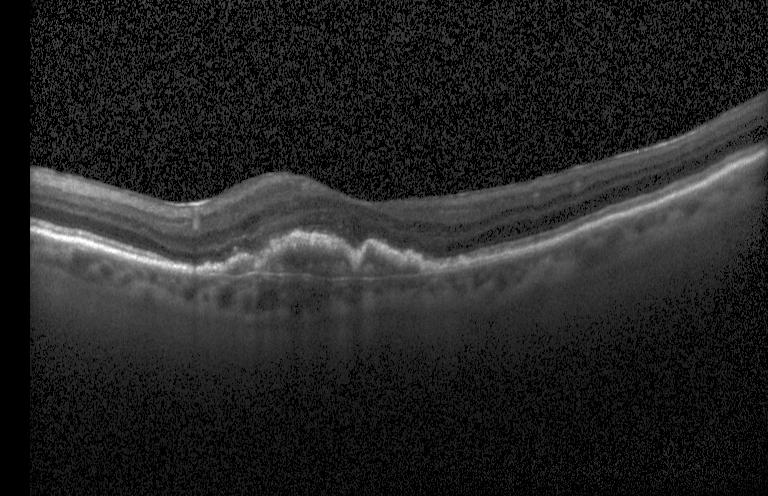 Retinal OCT B-scan; macular scan; acquired on a Heidelberg Spectralis — This B-scan demonstrates a choroidal neovascular membrane.